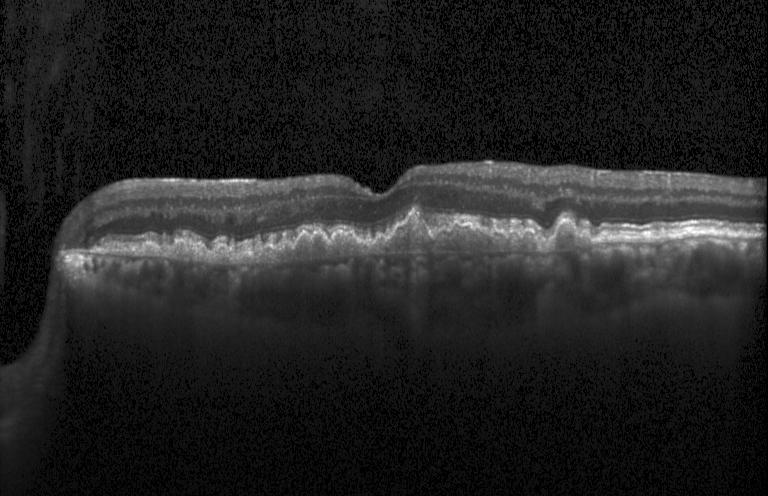

Optical coherence tomography scan. Instrument: Heidelberg Spectralis
Assessment: a choroidal neovascular membrane.